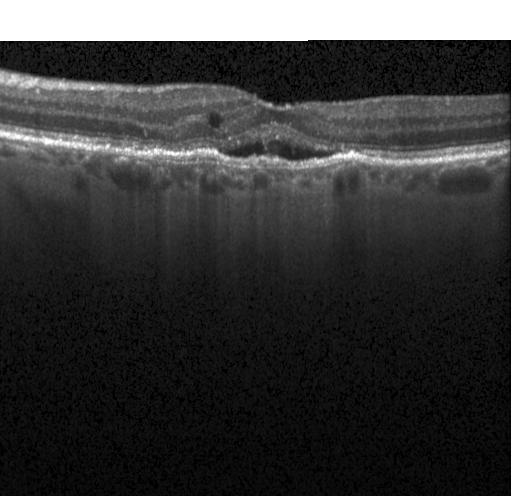
Spectral-domain optical coherence tomography · fovea-centered · instrument: Heidelberg Spectralis · retinal OCT cross-section. Diagnosis: a choroidal neovascular membrane.